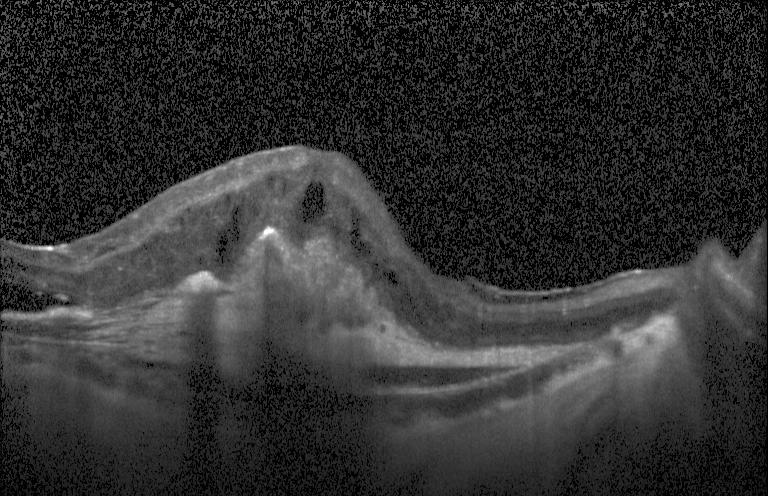 Macular OCT: a choroidal neovascular membrane.